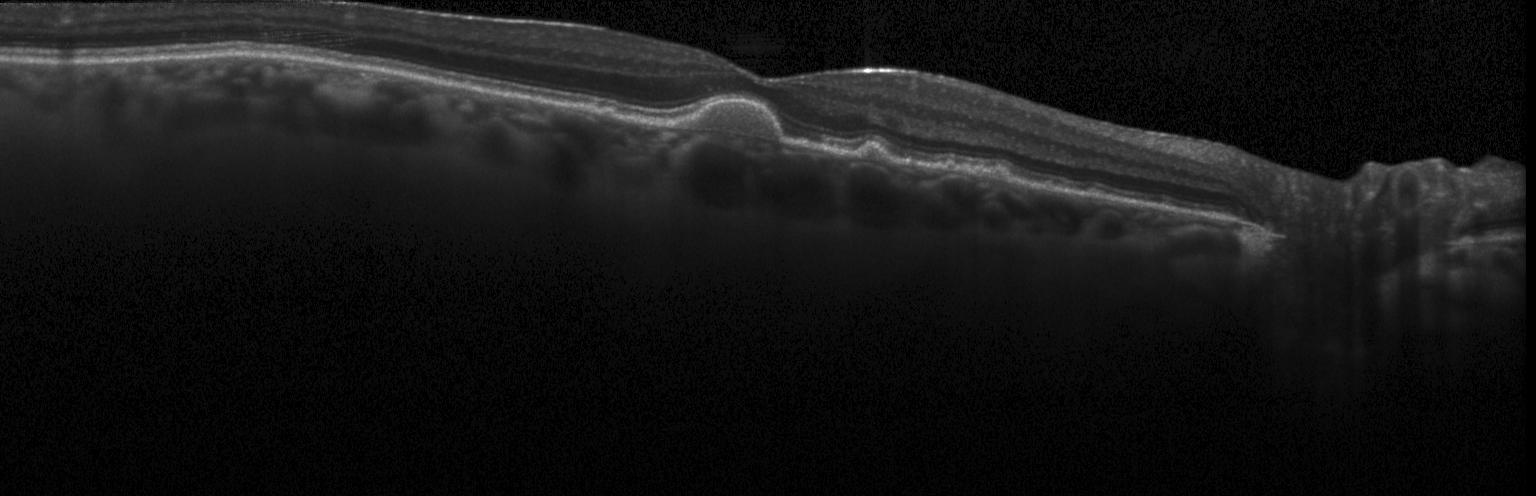

Macular OCT demonstrating drusen.